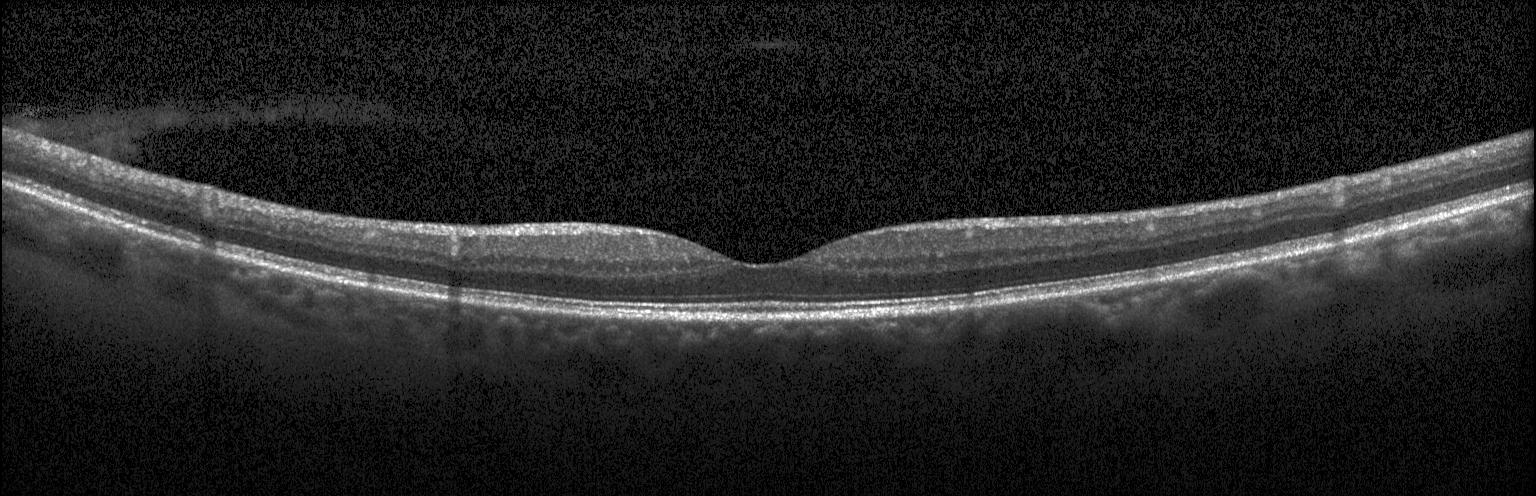 Impression: neither CNV, DME, nor drusen.